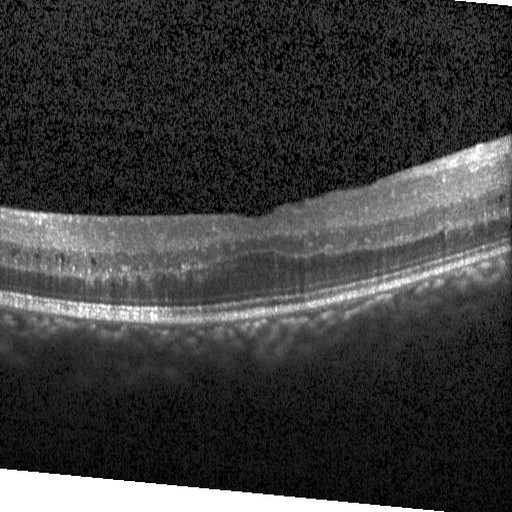
Spectral-domain OCT. Heidelberg Spectralis. Macular scan. Optical coherence tomography scan. Assessment: diabetic macular edema.